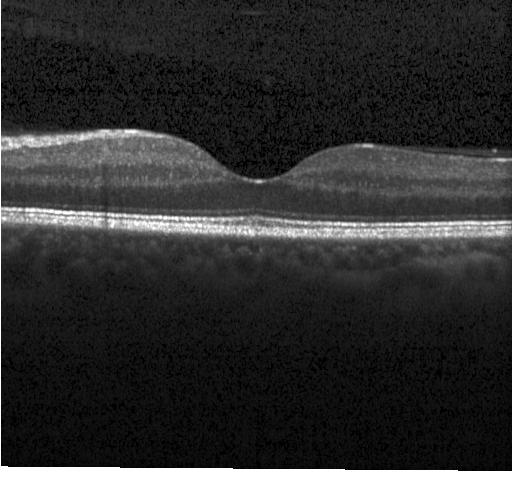 Impression: no choroidal neovascularization, no diabetic macular edema, and no drusen.